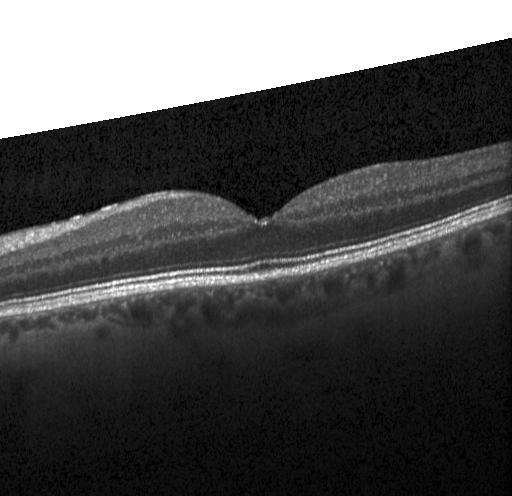 Optical coherence tomography scan · horizontal scan through the fovea · acquired on a Heidelberg Spectralis · spectral-domain OCT
Diagnosis: no CNV, no DME, and no drusen.